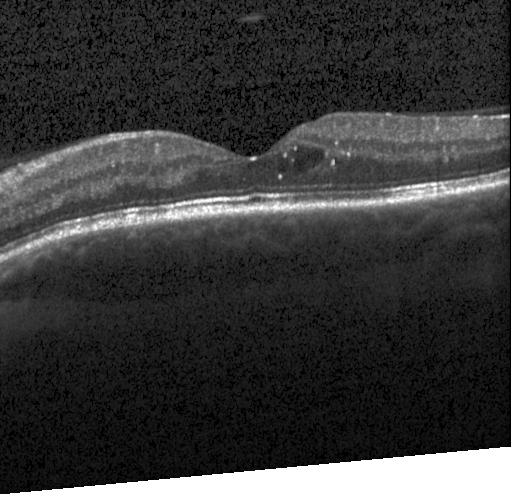

OCT line scan, horizontal scan through the fovea. Dx: DME.